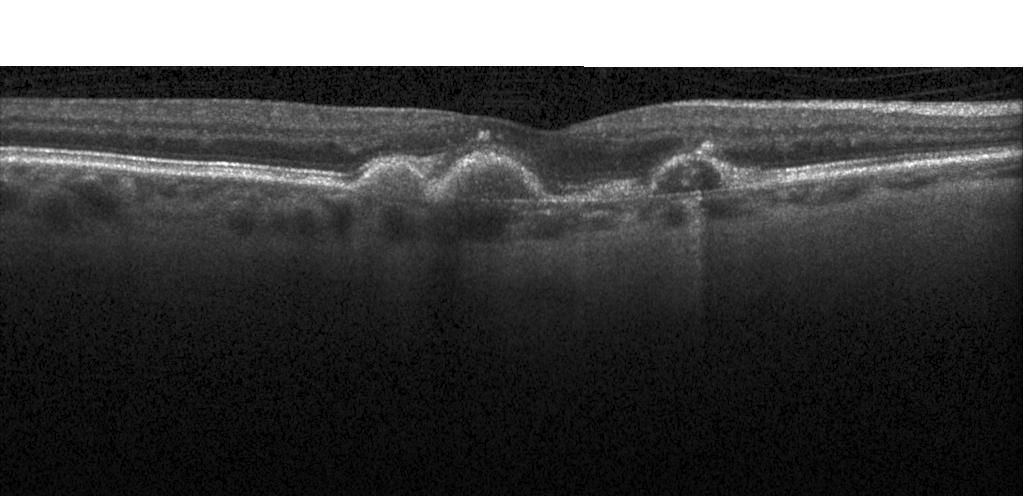
Through the macula, optical coherence tomography scan. Finding: a choroidal neovascular membrane.